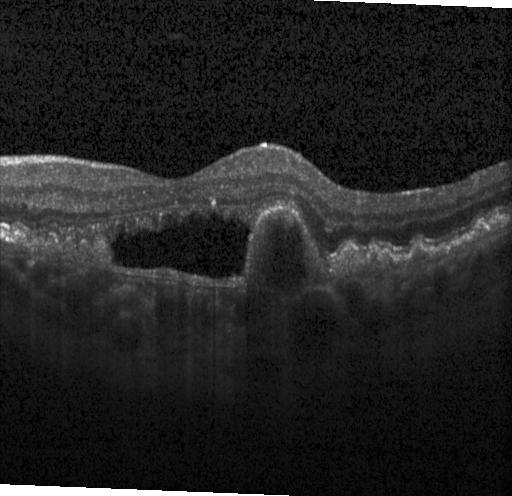
Finding: CNV.